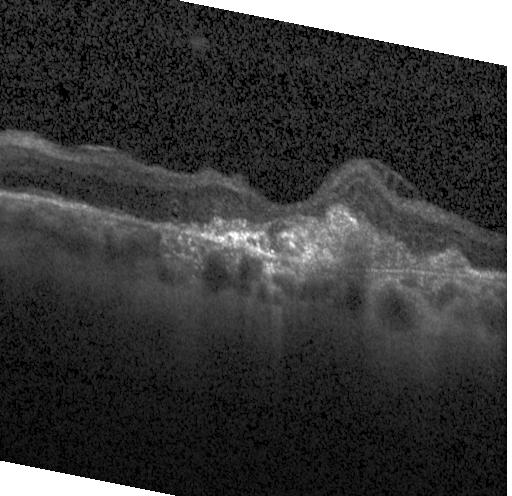
Optical coherence tomography B-scan.
The scan shows a choroidal neovascular membrane.